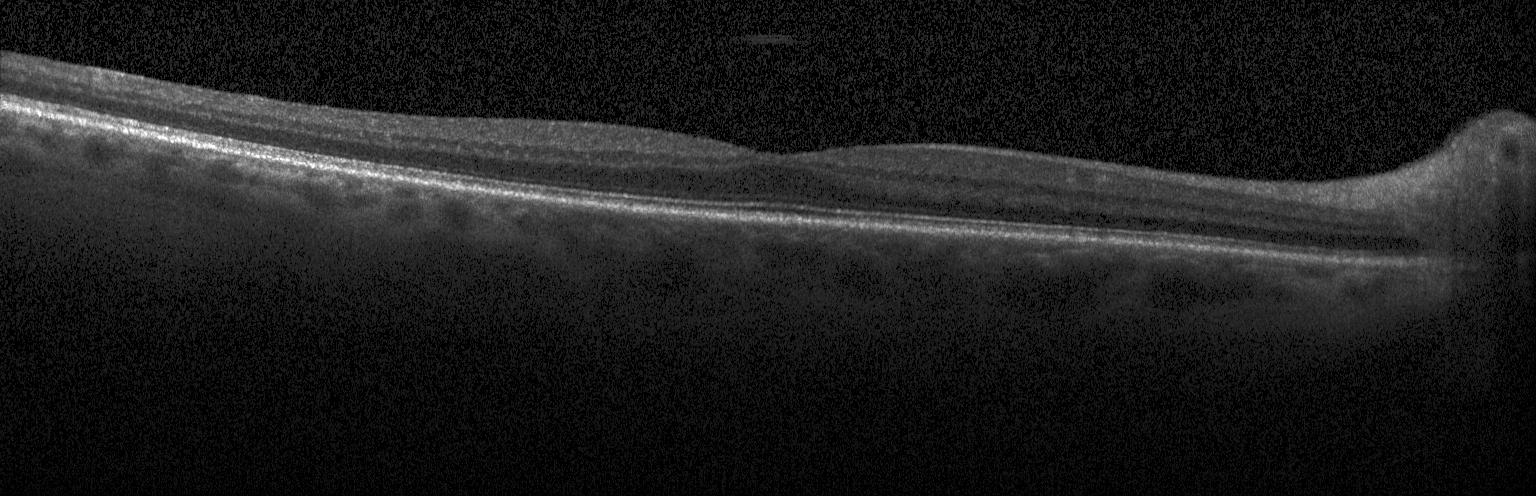

Instrument: Heidelberg Spectralis, retinal OCT cross-section, fovea-centered, SD-OCT.
Assessment: no choroidal neovascularization, no diabetic macular edema, and no drusen.